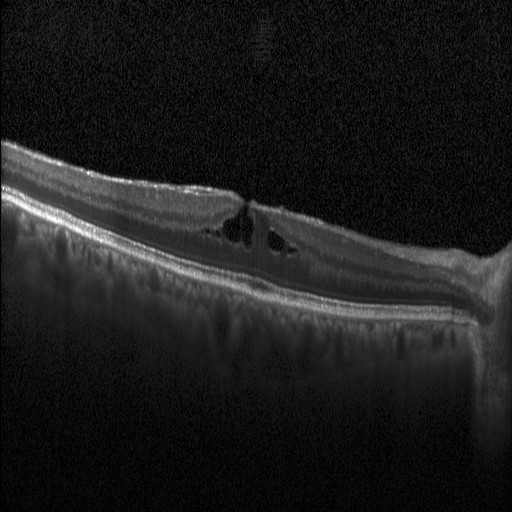

Finding: DME.